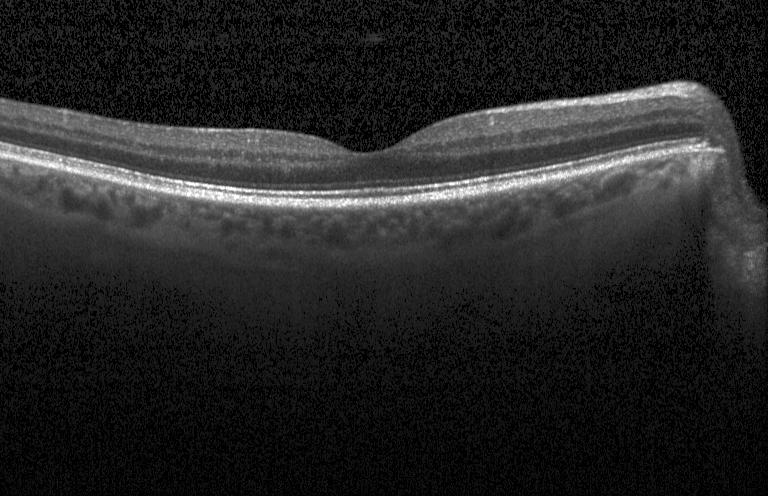

Assessment: no choroidal neovascularization, diabetic macular edema, or drusen.